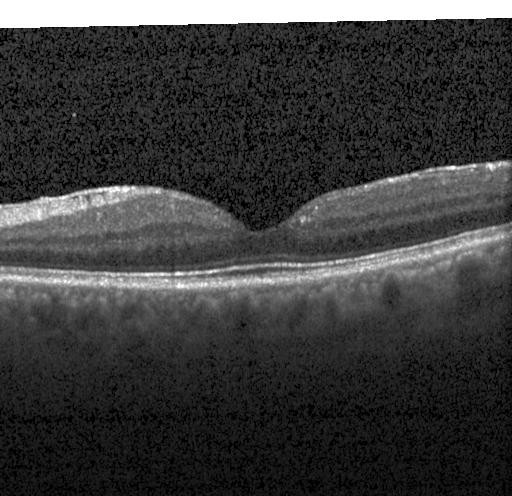

Retinal OCT cross-section — Assessment: no evidence of CNV, DME, or drusen.